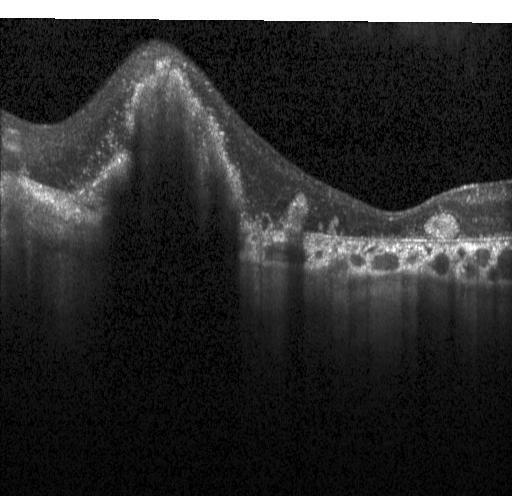
The scan shows CNV.